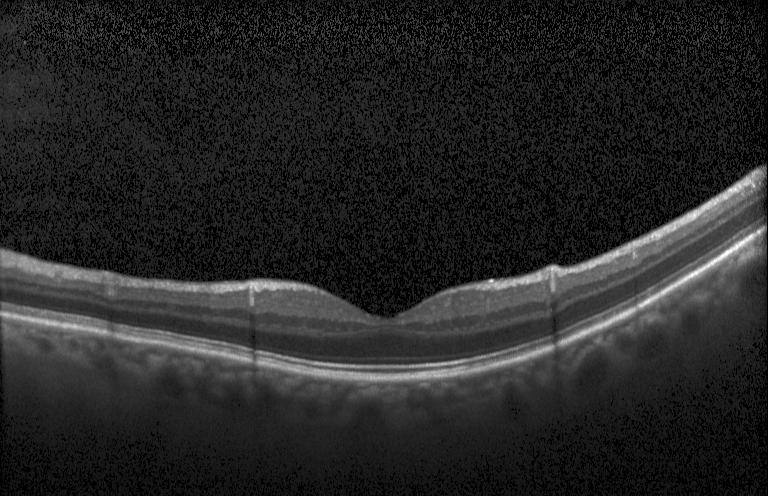
Through the macula, SD-OCT, retinal OCT B-scan. Impression: neither choroidal neovascularization, diabetic macular edema, nor drusen.